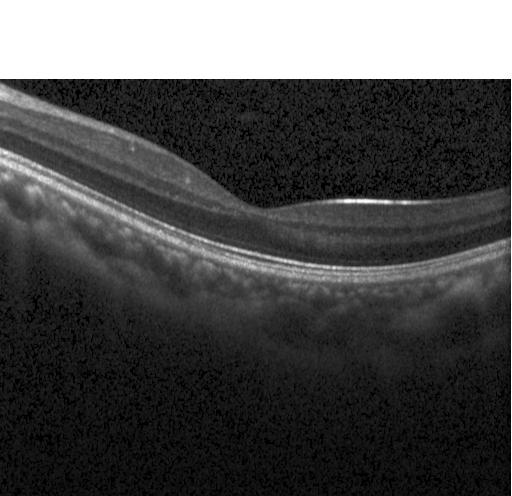
Optical coherence tomography B-scan · macular scan · SD-OCT
Neither choroidal neovascularization, diabetic macular edema, nor drusen.